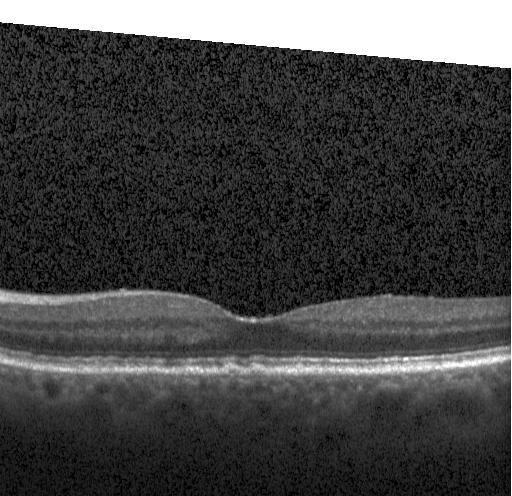
Optical coherence tomography B-scan
Finding: sub-RPE drusenoid deposits.